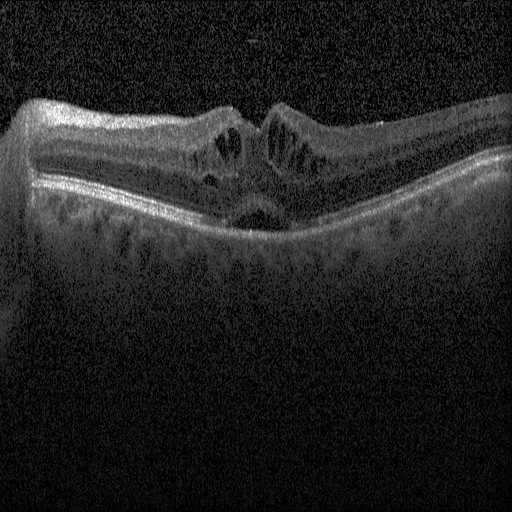
Instrument: Heidelberg Spectralis; retinal OCT cross-section
Assessment: diabetic macular edema.